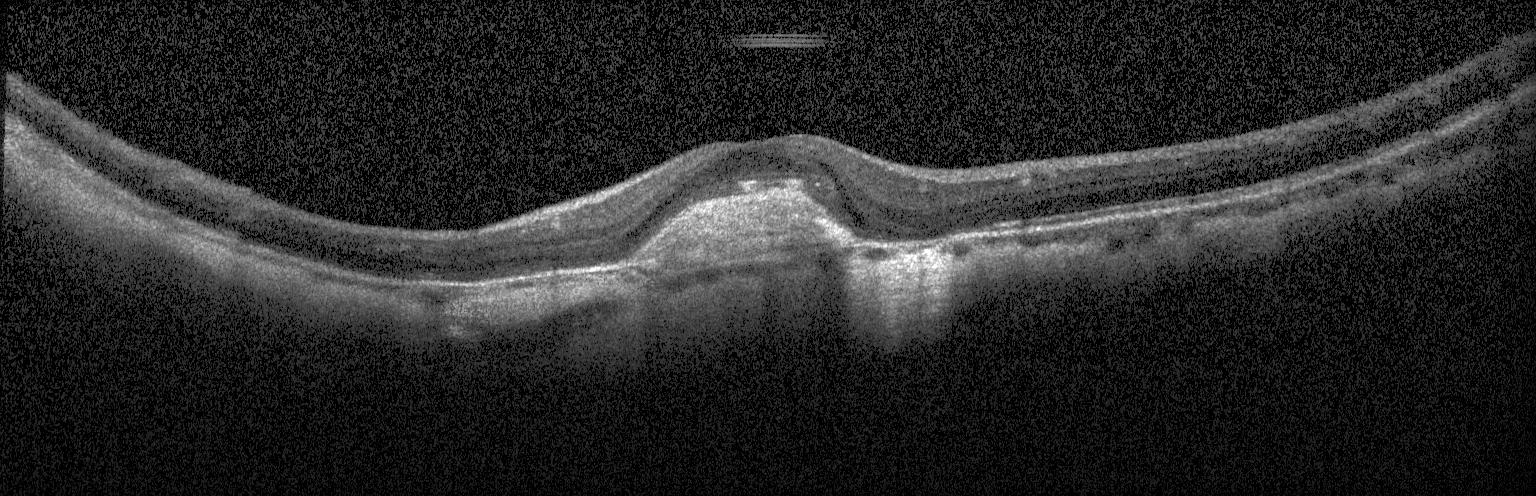 Horizontal scan through the fovea · Heidelberg Spectralis · spectral-domain OCT · optical coherence tomography B-scan
Dx: choroidal neovascularization (CNV).